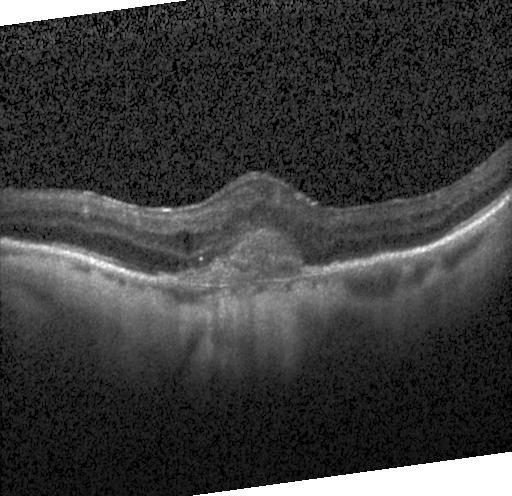 Macular OCT: choroidal neovascularization.